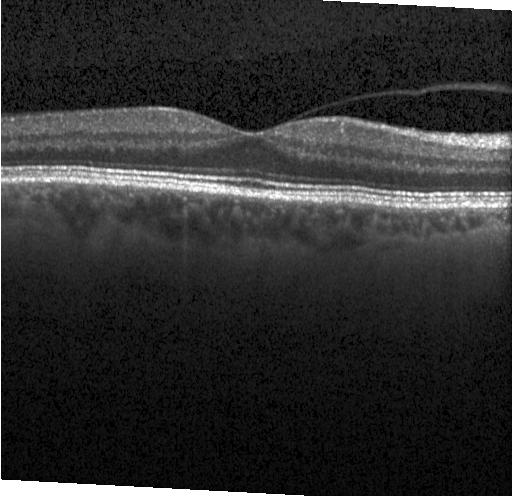
OCT B-scan, acquired on a Heidelberg Spectralis, through the macula — This B-scan demonstrates no evidence of CNV, DME, or drusen.